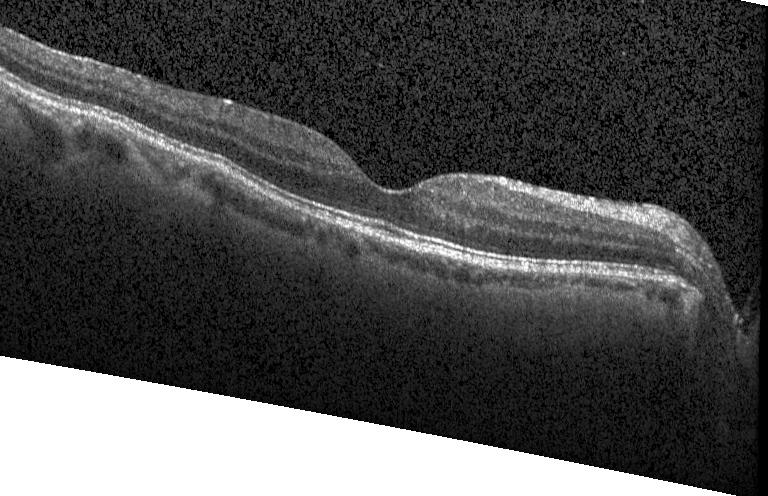
The scan shows no choroidal neovascularization, no diabetic macular edema, and no drusen.